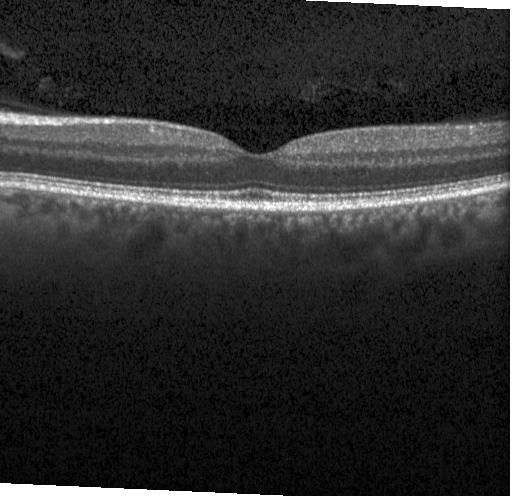 OCT finding: no CNV, DME, or drusen.